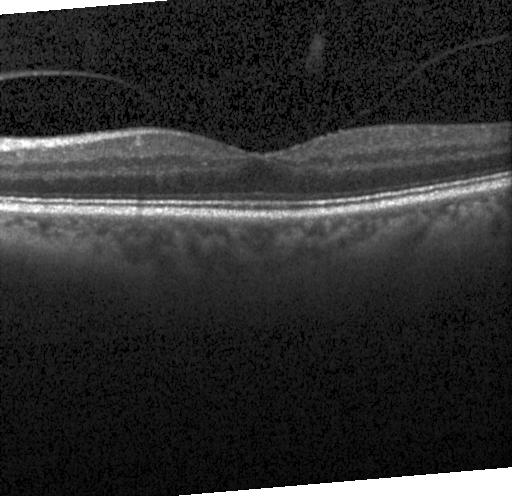
Centered on the fovea, Heidelberg Spectralis, optical coherence tomography scan, spectral-domain optical coherence tomography
OCT finding: neither choroidal neovascularization, diabetic macular edema, nor drusen.